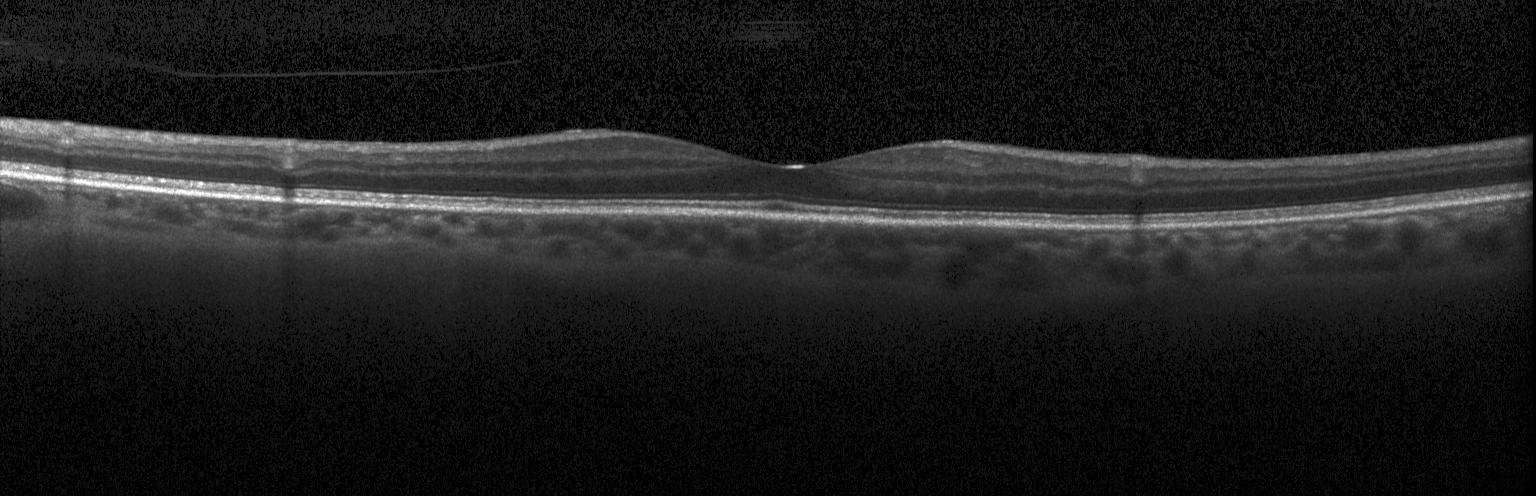
Retinal OCT cross-section showing neither CNV, DME, nor drusen.